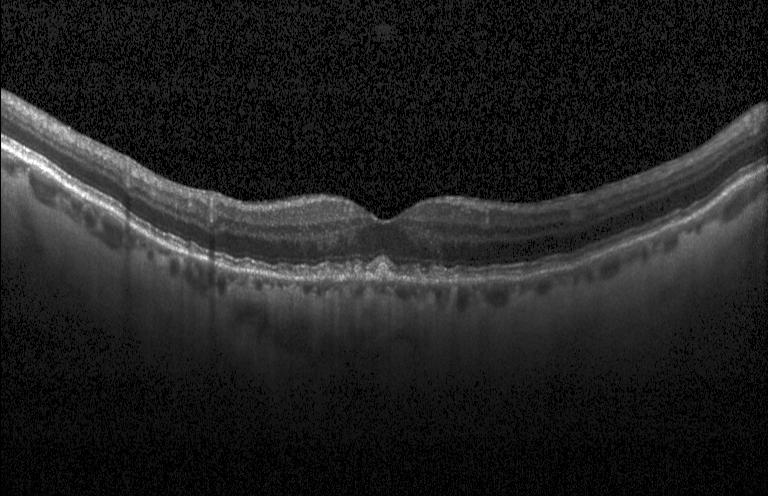
Finding: sub-RPE drusenoid deposits.